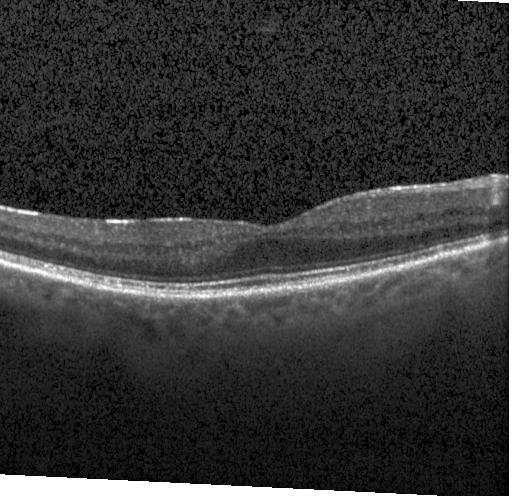
No choroidal neovascularization, diabetic macular edema, or drusen.